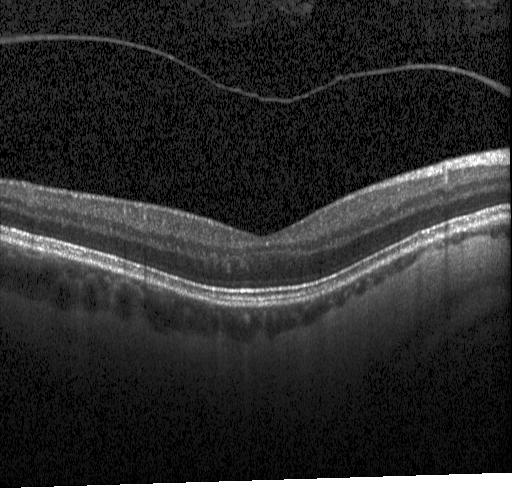
Retinal OCT cross-section
Impression: no choroidal neovascularization, no diabetic macular edema, and no drusen.